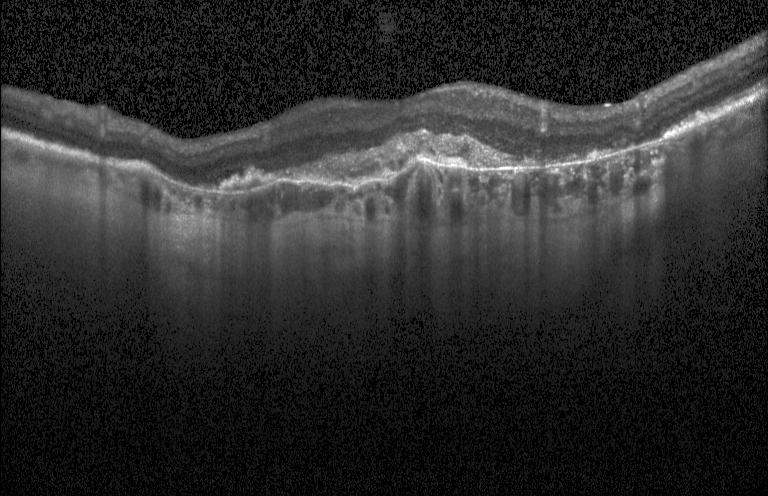

Diagnosis: choroidal neovascularization (CNV).